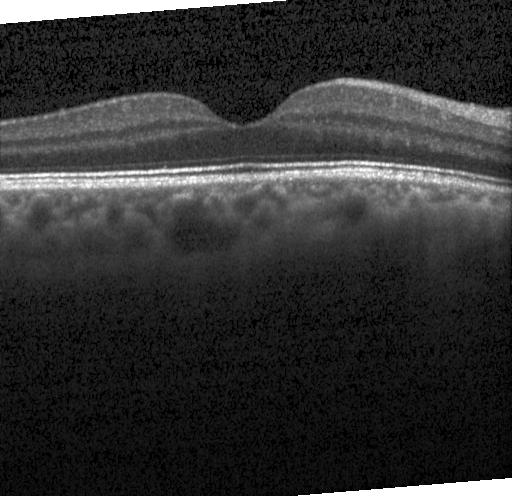 Dx: no CNV, DME, or drusen.